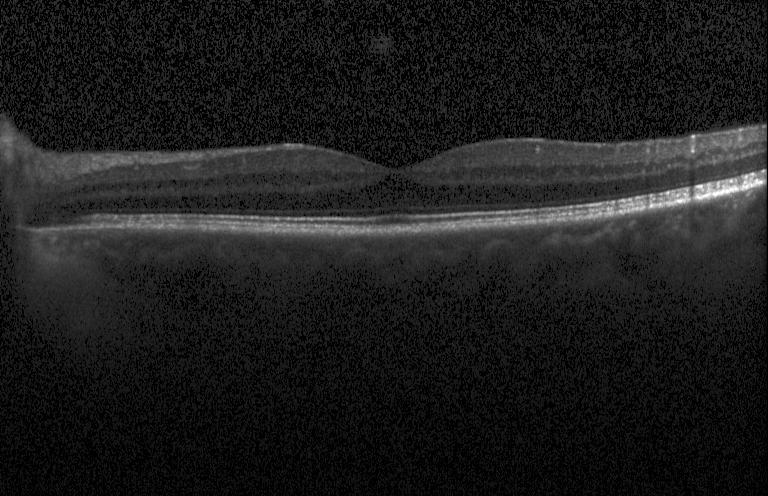

Optical coherence tomography scan. Heidelberg Spectralis OCT system. Horizontal scan through the fovea — Finding: no evidence of choroidal neovascularization, diabetic macular edema, or drusen.